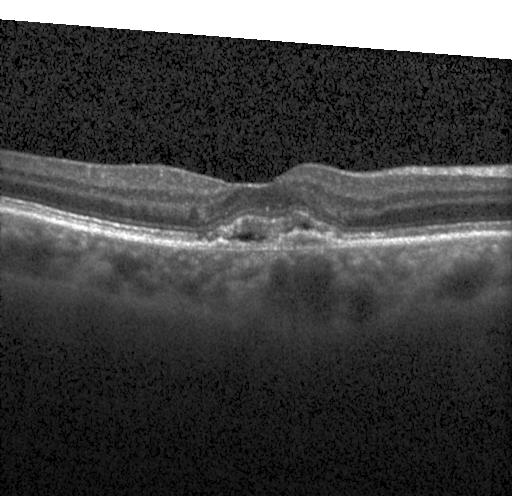

OCT B-scan — OCT finding: a choroidal neovascular membrane.